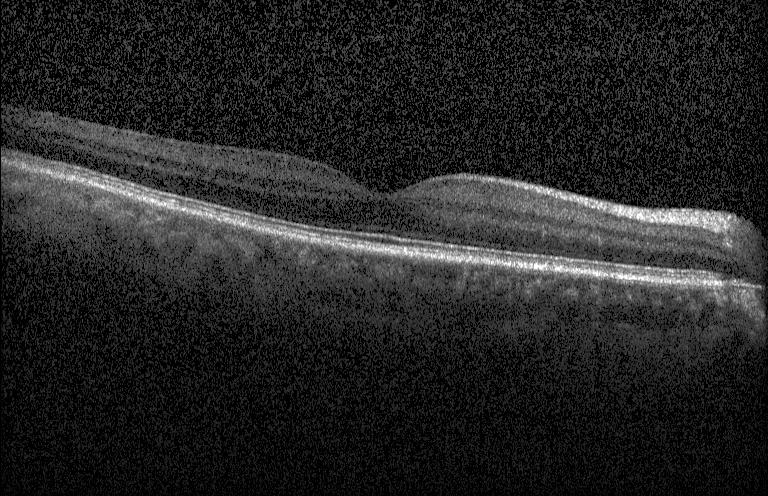 Diagnosis: neither CNV, DME, nor drusen.